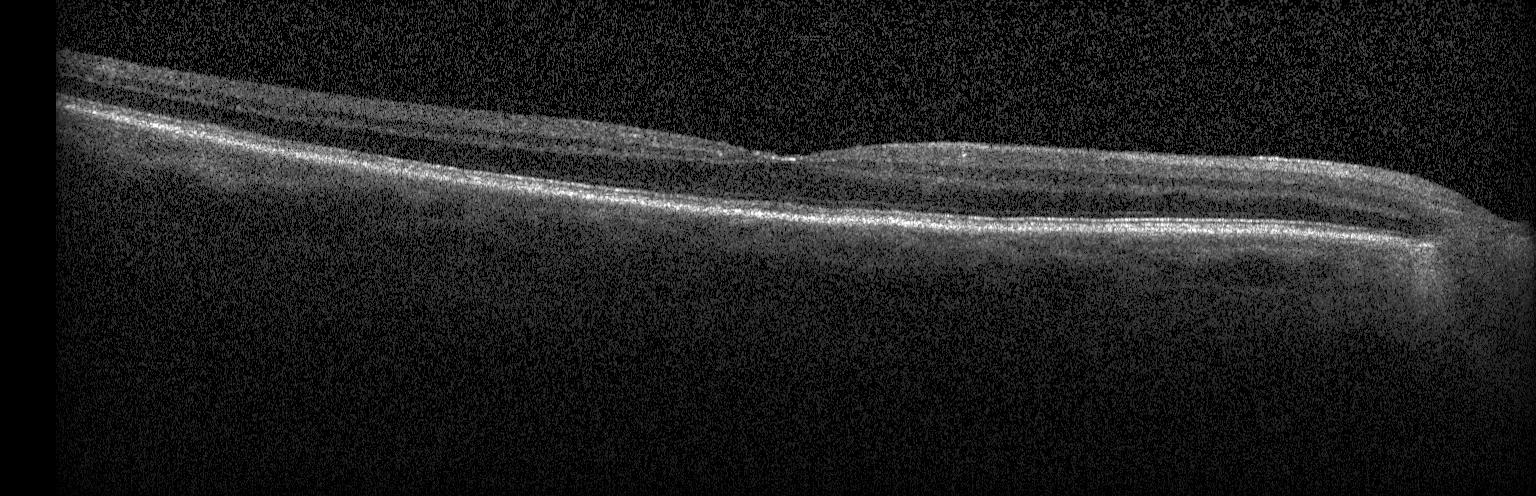

No choroidal neovascularization, no diabetic macular edema, and no drusen.